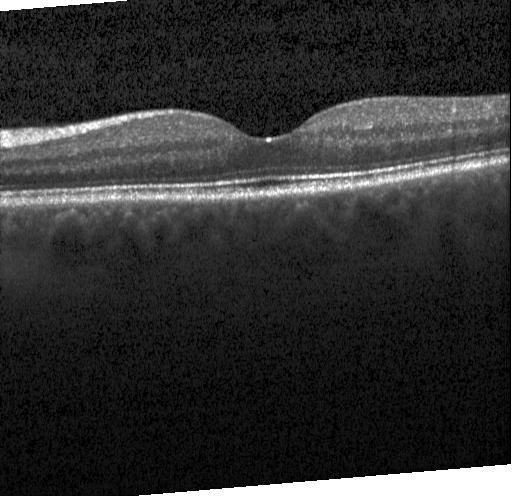
OCT scan showing no evidence of choroidal neovascularization, diabetic macular edema, or drusen.